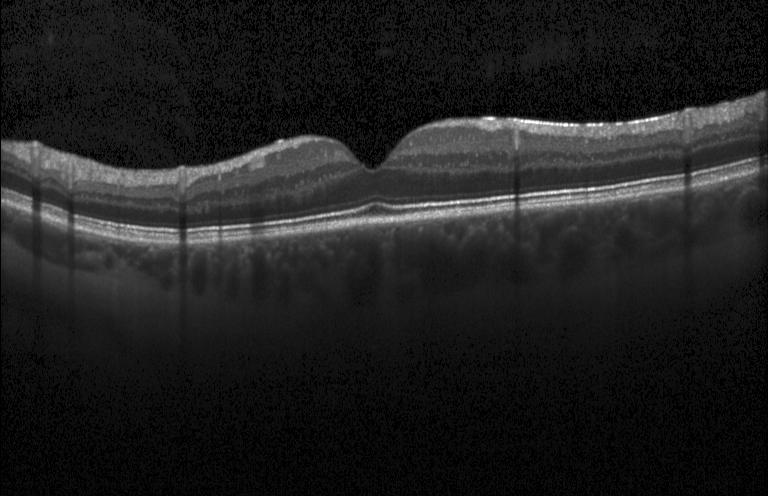 Retinal OCT B-scan. OCT finding: no choroidal neovascularization, diabetic macular edema, or drusen.